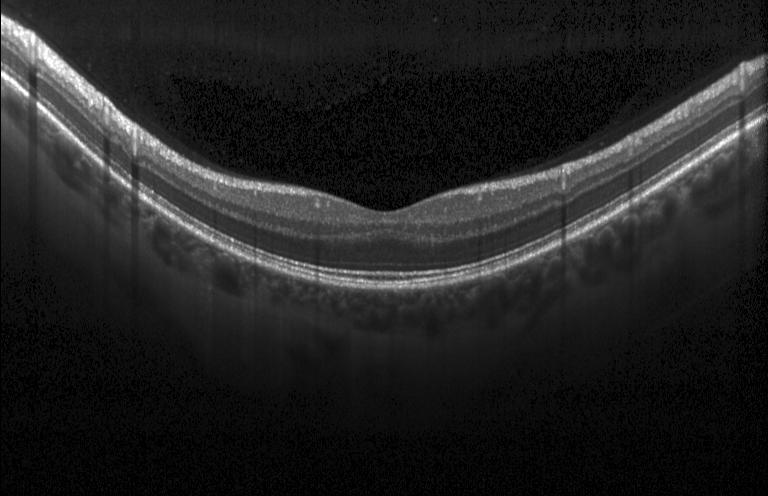

Retinal OCT cross-section showing no choroidal neovascularization, no diabetic macular edema, and no drusen.